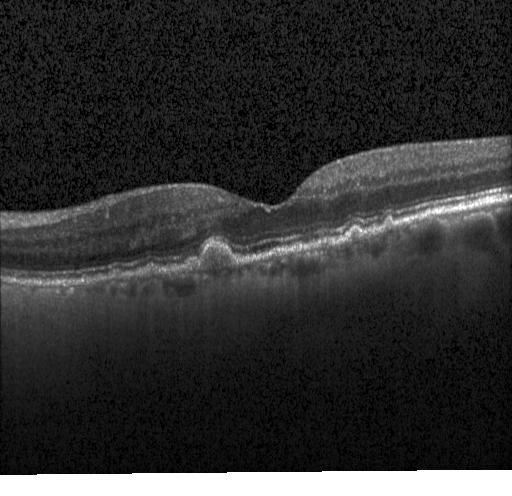
Impression: multiple drusen.